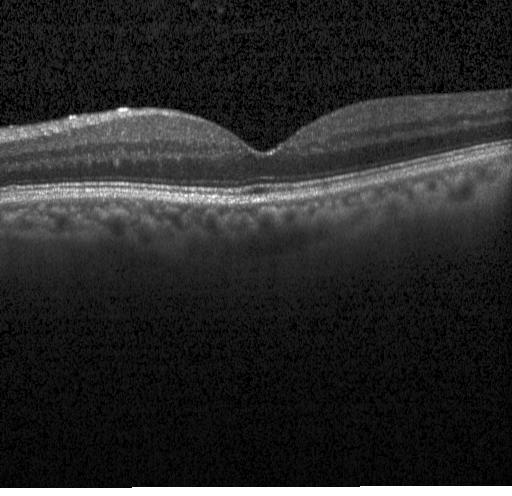

Spectral-domain optical coherence tomography. Horizontal scan through the fovea. Retinal OCT cross-section. Acquired on a Heidelberg Spectralis — Dx: no evidence of choroidal neovascularization, diabetic macular edema, or drusen.